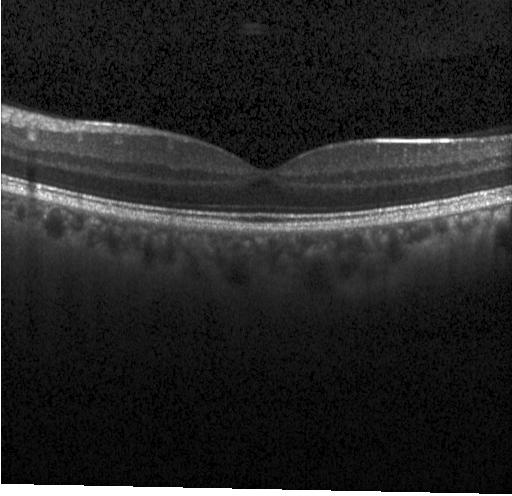 Retinal OCT B-scan — The scan shows no evidence of CNV, DME, or drusen.